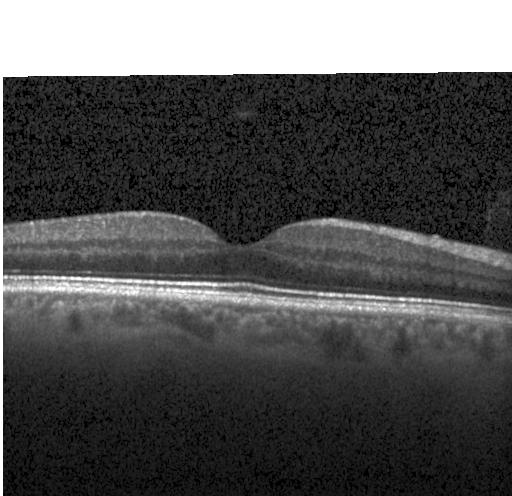
OCT finding: neither CNV, DME, nor drusen.